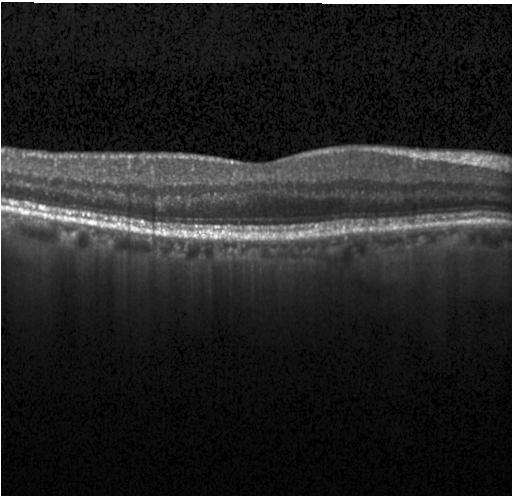
OCT finding: neither choroidal neovascularization, diabetic macular edema, nor drusen.